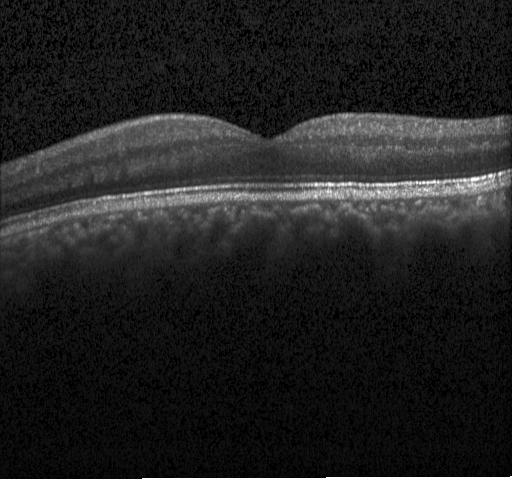

Through the macula. Heidelberg Spectralis OCT system. OCT line scan
Finding: no choroidal neovascularization, diabetic macular edema, or drusen.